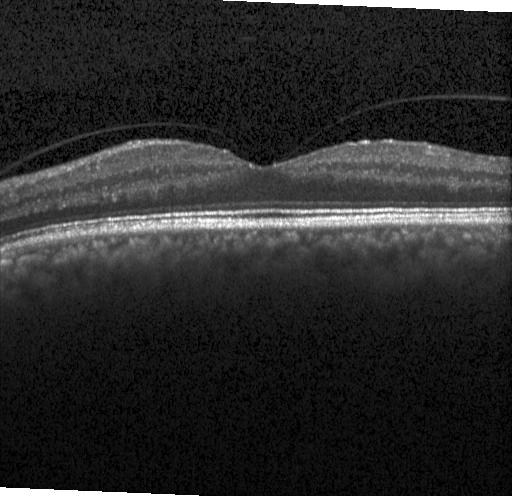

OCT finding: no choroidal neovascularization, no diabetic macular edema, and no drusen.